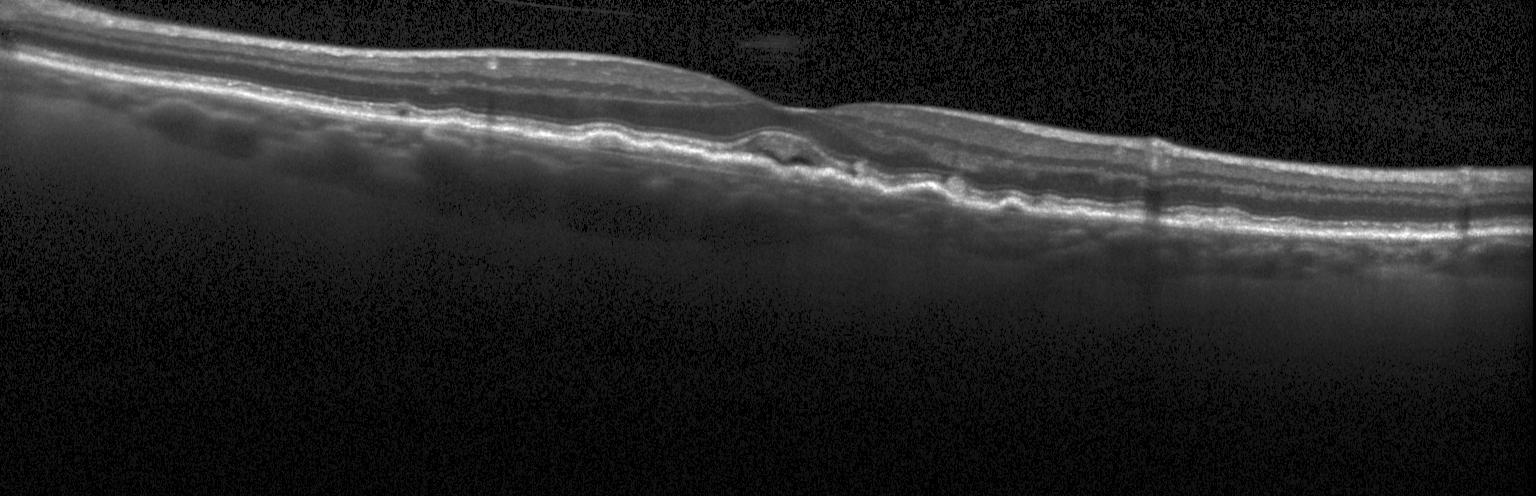 SD-OCT; optical coherence tomography scan; instrument: Heidelberg Spectralis.
Choroidal neovascularization (CNV).